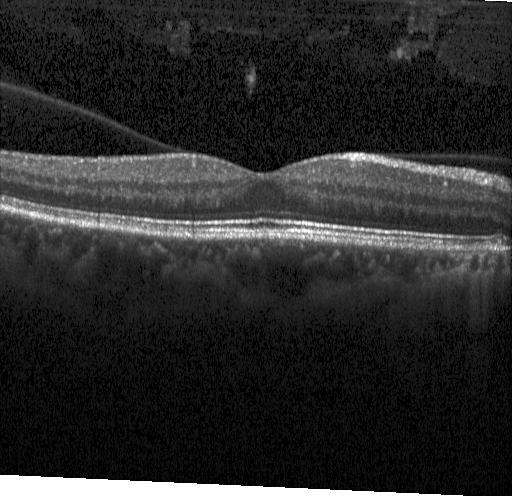

This B-scan demonstrates neither choroidal neovascularization, diabetic macular edema, nor drusen.